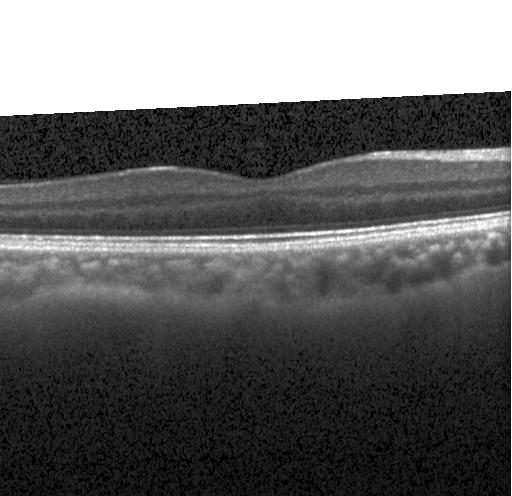

OCT B-scan.
Dx: no choroidal neovascularization, diabetic macular edema, or drusen.